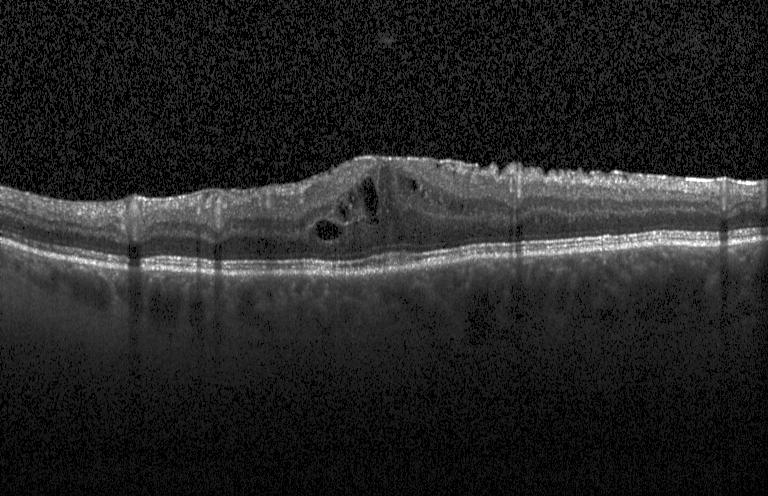
Centered on the fovea. Spectral-domain OCT. Acquired on a Heidelberg Spectralis. Retinal OCT B-scan — Diagnosis: DME.